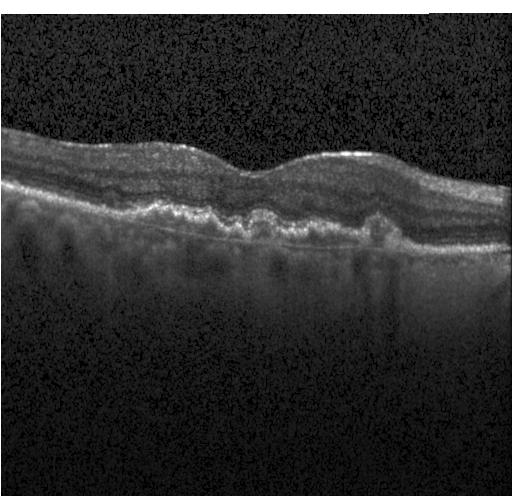

Horizontal scan through the fovea. Instrument: Heidelberg Spectralis. Spectral-domain OCT. Optical coherence tomography scan — Impression: a choroidal neovascular membrane.